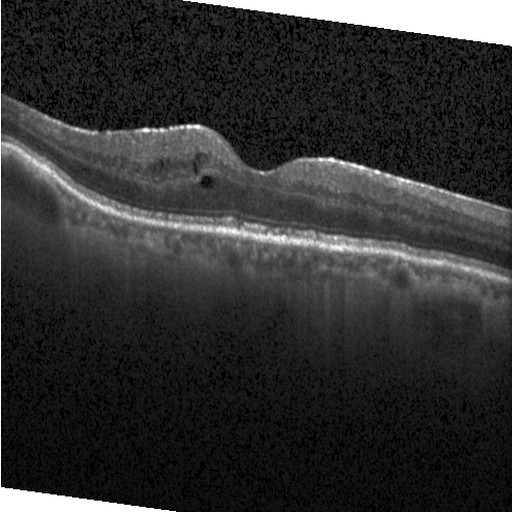

The scan shows diabetic macular edema (DME).